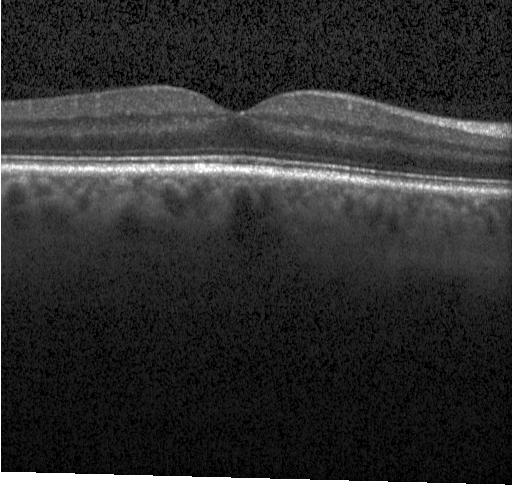
Macular OCT: neither choroidal neovascularization, diabetic macular edema, nor drusen.